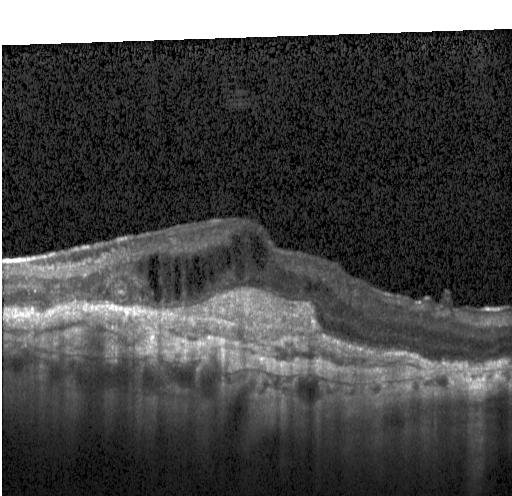 Heidelberg Spectralis OCT system; retinal OCT B-scan. Impression: choroidal neovascularization (CNV).